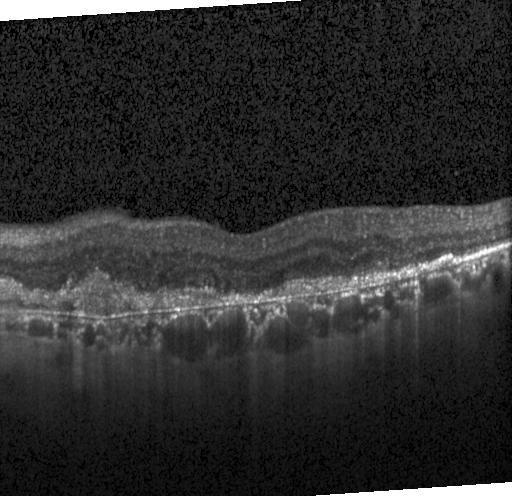

Heidelberg Spectralis, retinal OCT cross-section — Impression: choroidal neovascularization (CNV).